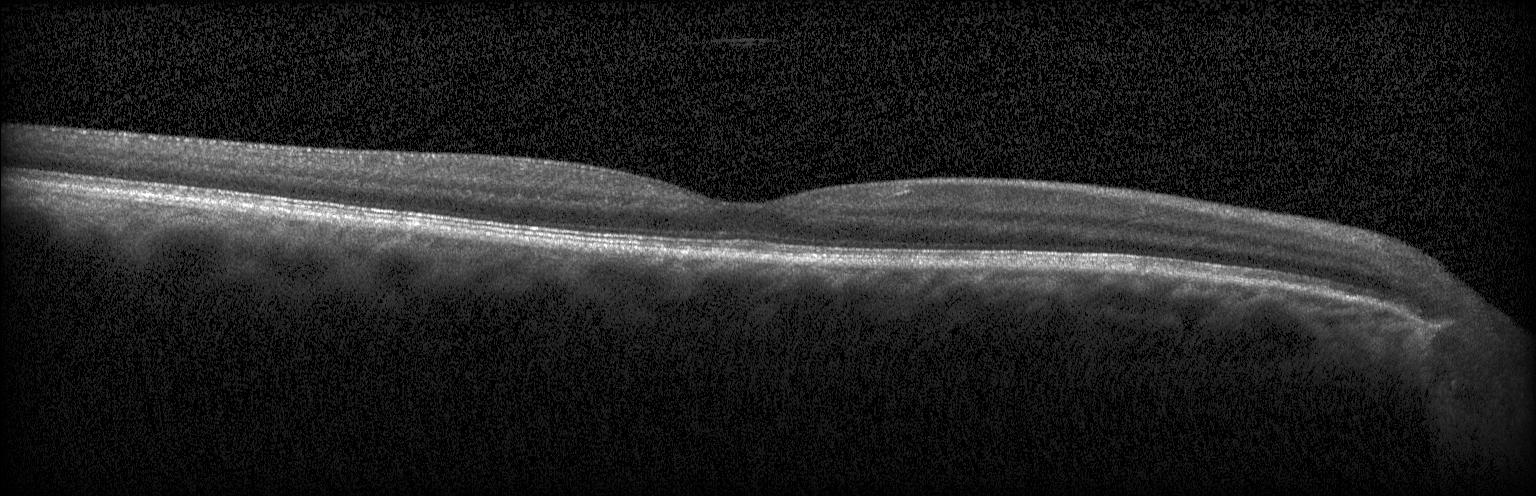 Optical coherence tomography B-scan; through the macula.
OCT finding: no CNV, no DME, and no drusen.